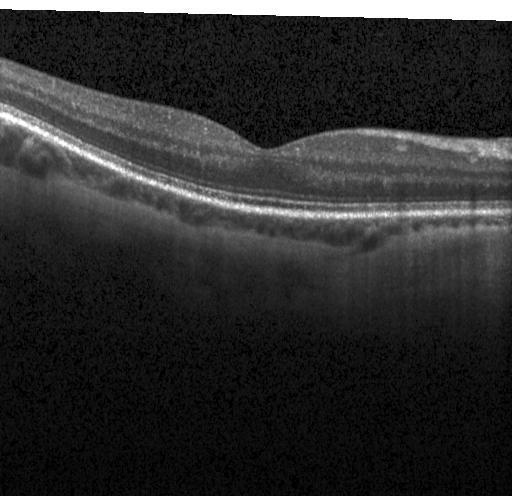 Optical coherence tomography scan. Macular OCT: no evidence of CNV, DME, or drusen.